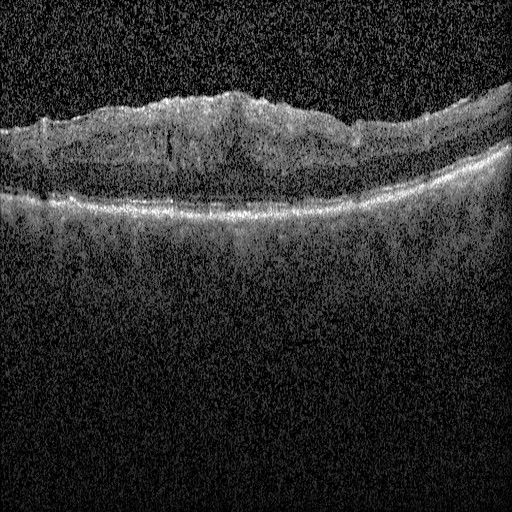
Impression: DME.